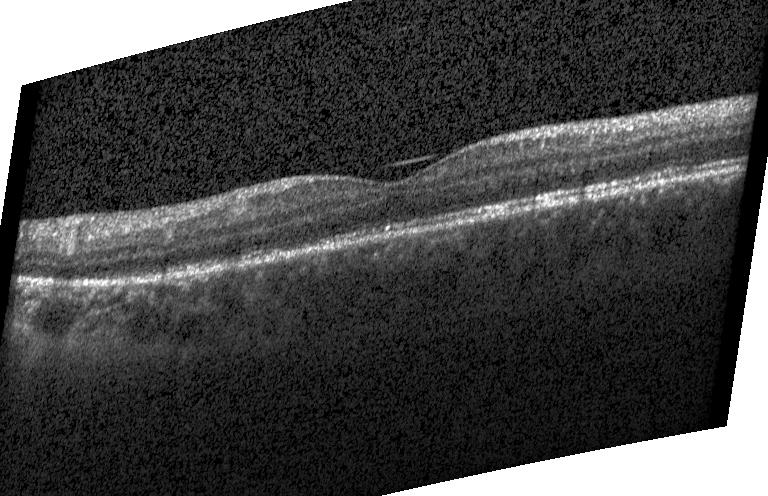

Dx: no CNV, DME, or drusen.